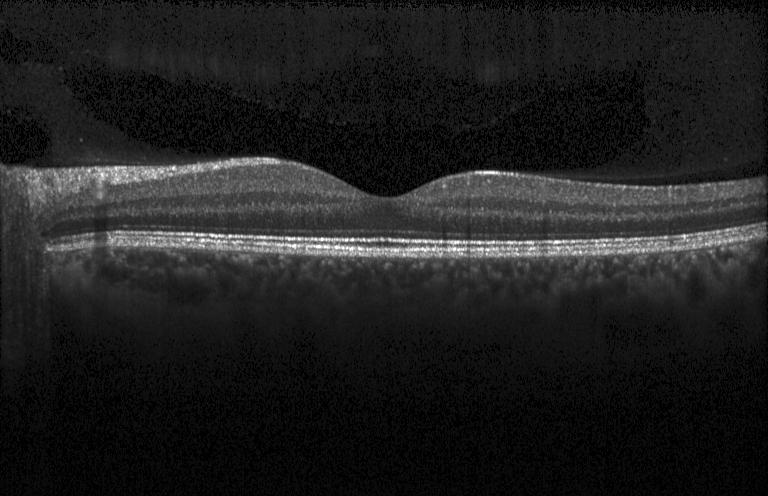

Finding: no choroidal neovascularization, no diabetic macular edema, and no drusen.